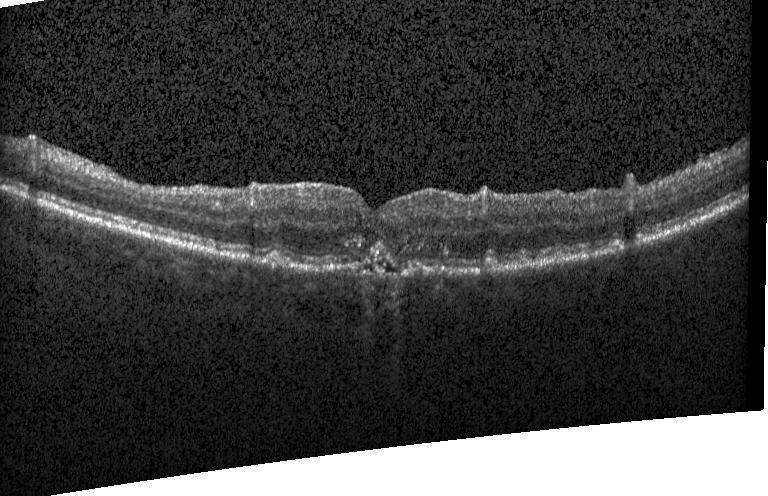
Retinal OCT B-scan; Heidelberg Spectralis. Impression: a choroidal neovascular membrane.